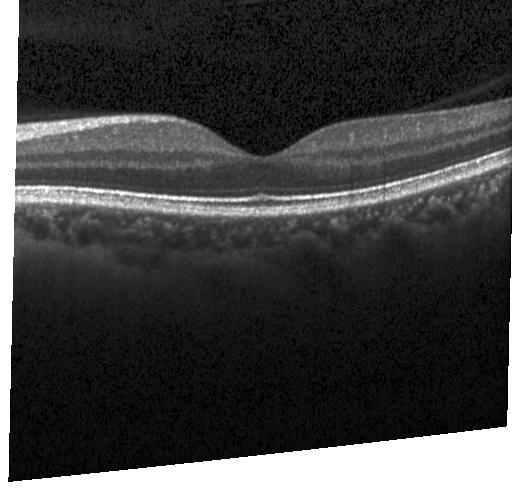 Retinal OCT B-scan — Finding: no evidence of choroidal neovascularization, diabetic macular edema, or drusen.